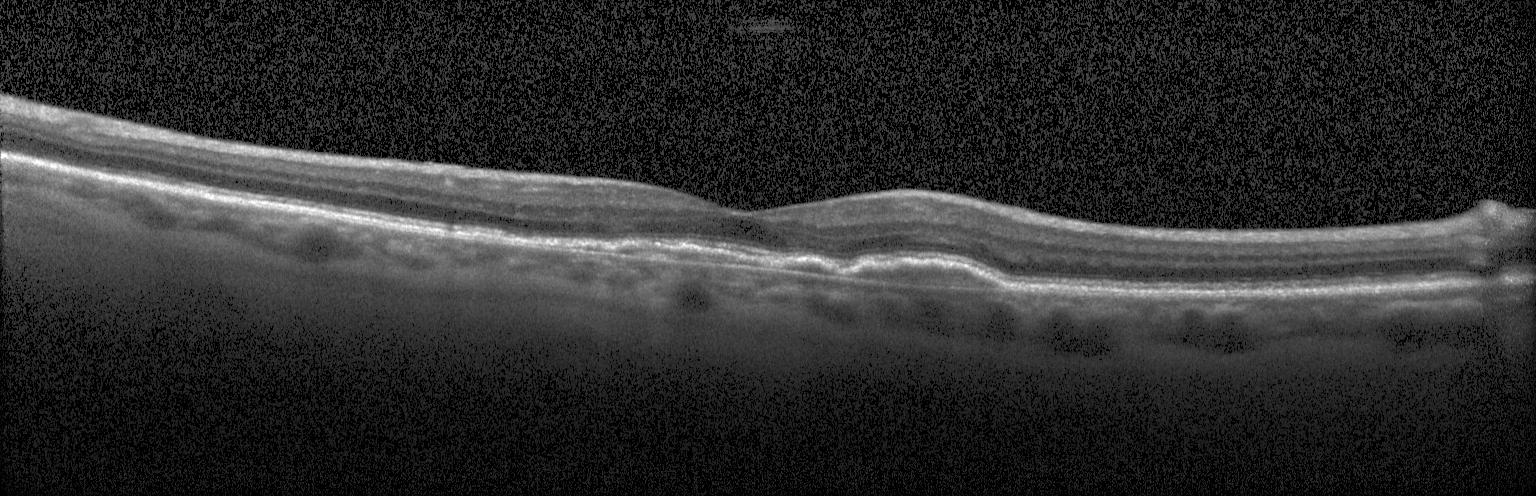 SD-OCT, Heidelberg Spectralis OCT system, retinal OCT cross-section, horizontal scan through the fovea. CNV.